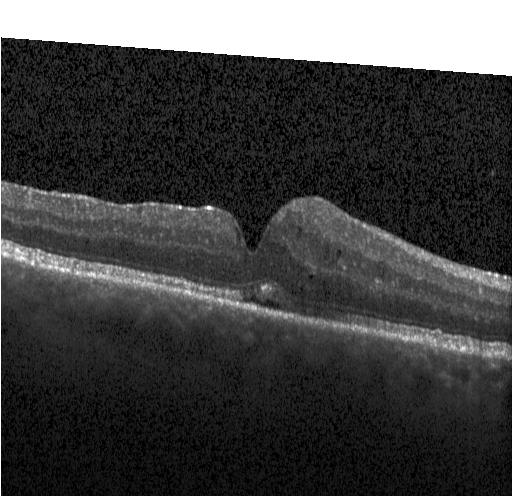 Retinal OCT cross-section; SD-OCT; instrument: Heidelberg Spectralis.
Assessment: DME.